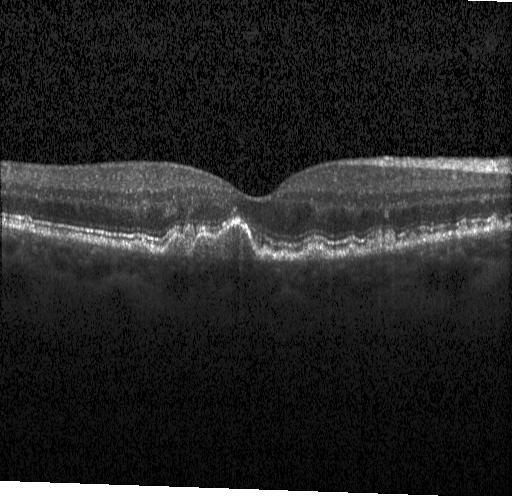 Impression: multiple drusen.